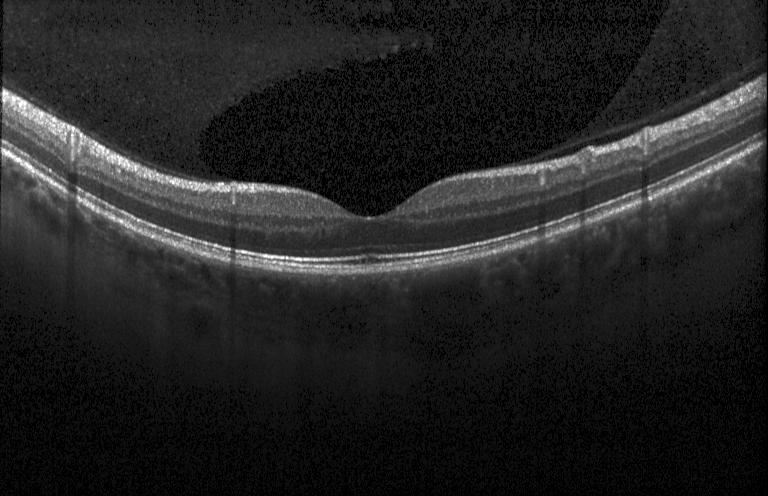
Dx: neither CNV, DME, nor drusen.